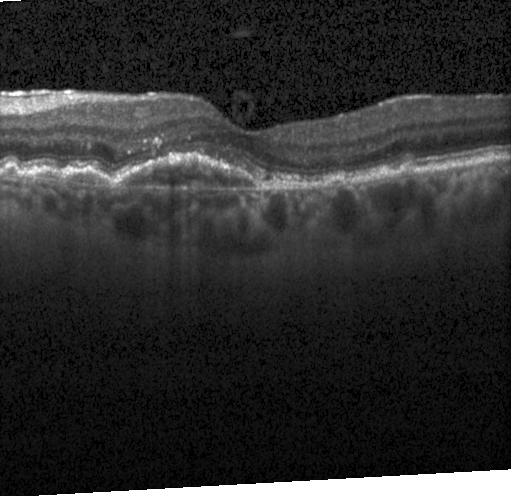 SD-OCT. Macular scan. OCT B-scan.
The scan shows CNV.